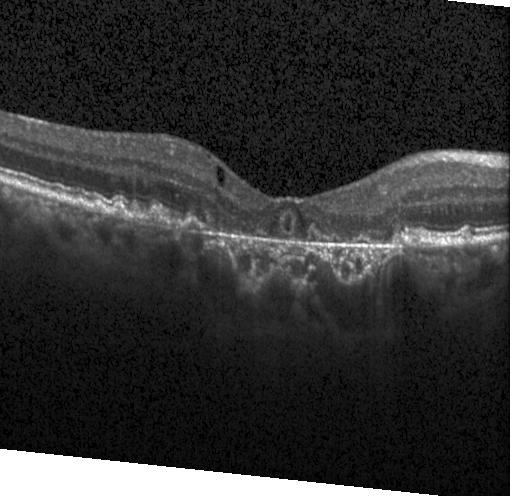

Optical coherence tomography B-scan. The scan shows a choroidal neovascular membrane.